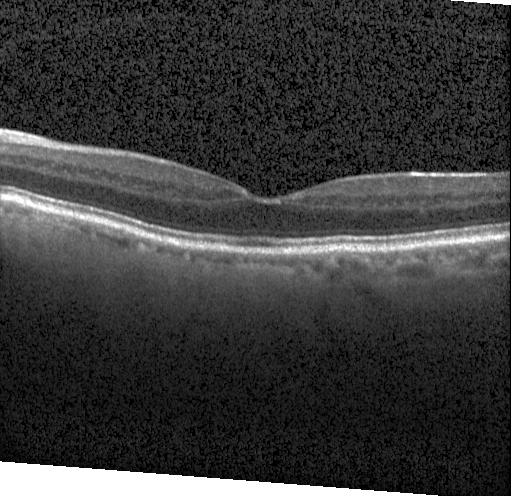 Impression: no evidence of choroidal neovascularization, diabetic macular edema, or drusen.